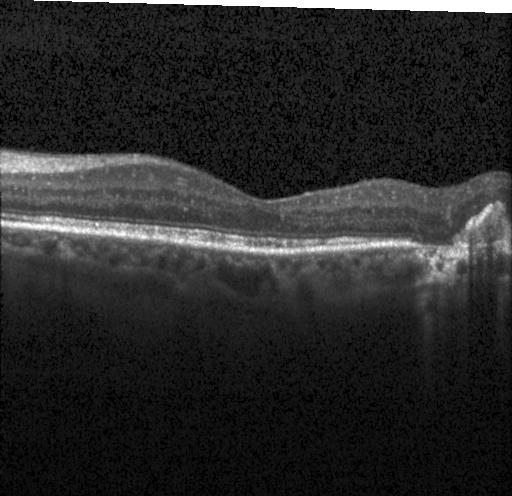 Spectral-domain OCT. OCT B-scan — Assessment: a choroidal neovascular membrane.